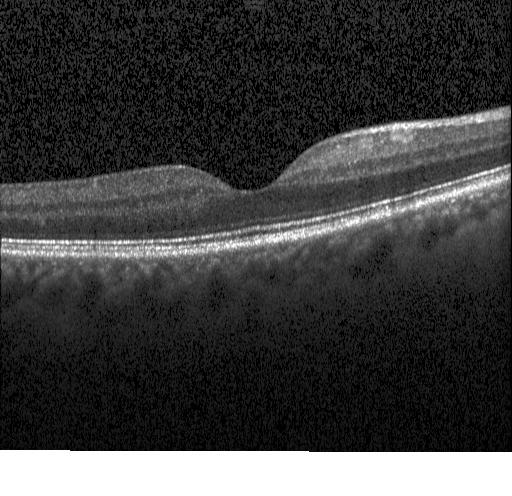 Macular OCT demonstrating no choroidal neovascularization, diabetic macular edema, or drusen.